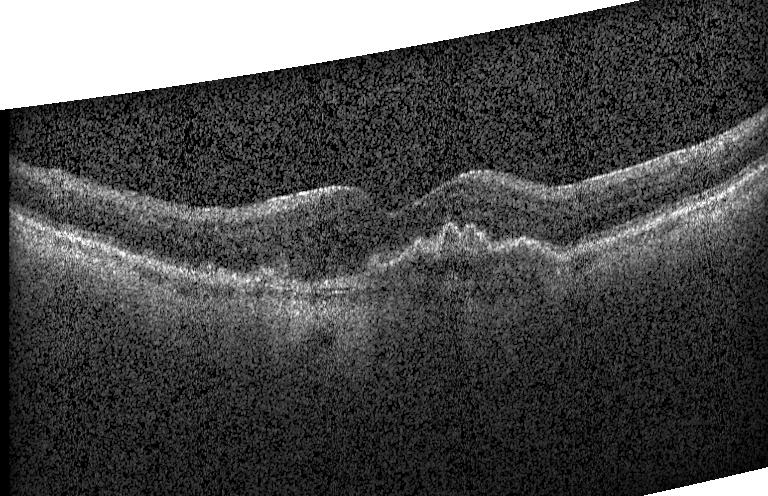
Macular OCT: choroidal neovascularization.